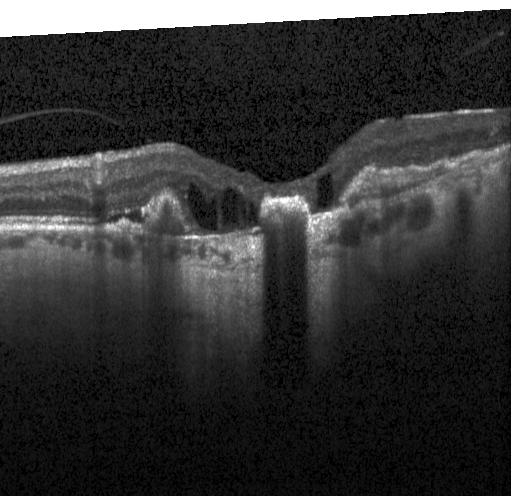

Dx: a choroidal neovascular membrane.